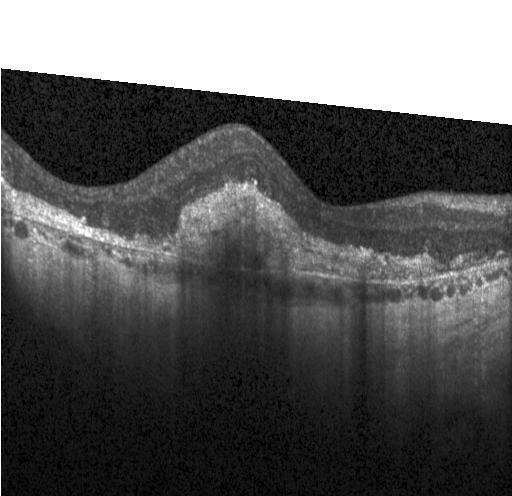

Retinal OCT cross-section showing choroidal neovascularization.